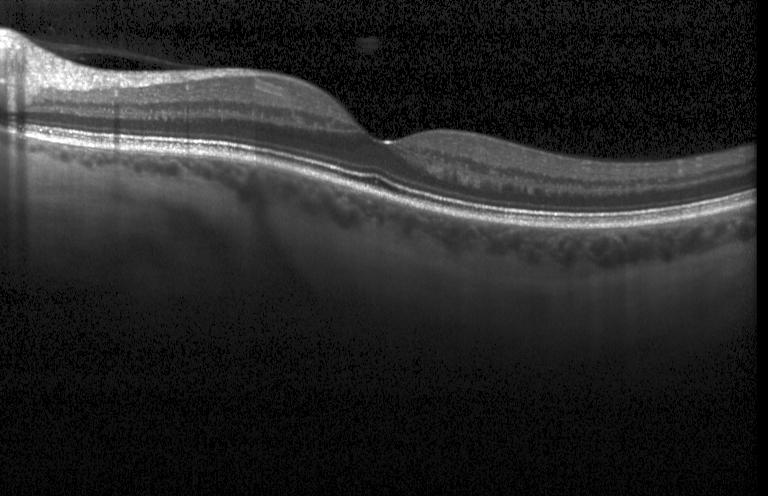

Heidelberg Spectralis, SD-OCT, OCT B-scan
Impression: no choroidal neovascularization, diabetic macular edema, or drusen.